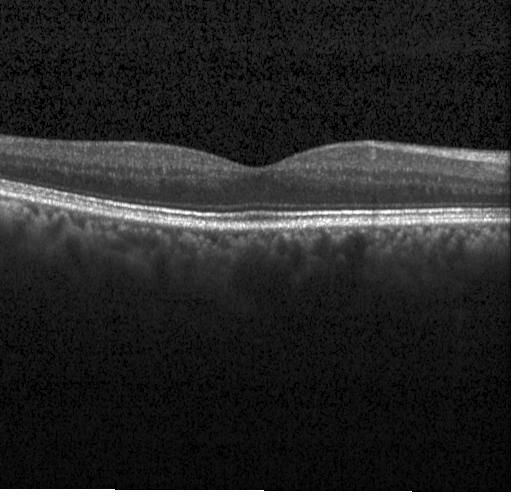

Acquired on a Heidelberg Spectralis, optical coherence tomography scan.
This B-scan demonstrates neither choroidal neovascularization, diabetic macular edema, nor drusen.